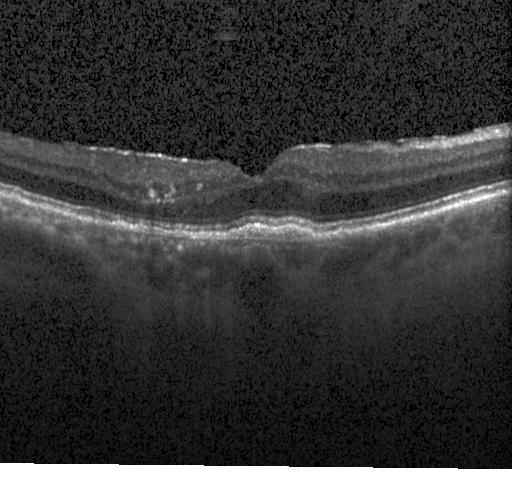
Diagnosis: a choroidal neovascular membrane.